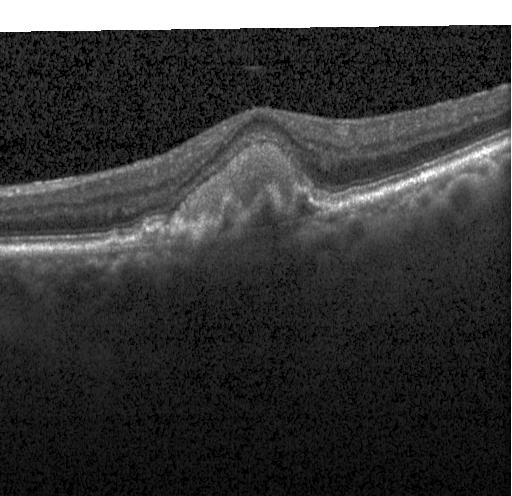 OCT B-scan
Diagnosis: choroidal neovascularization.